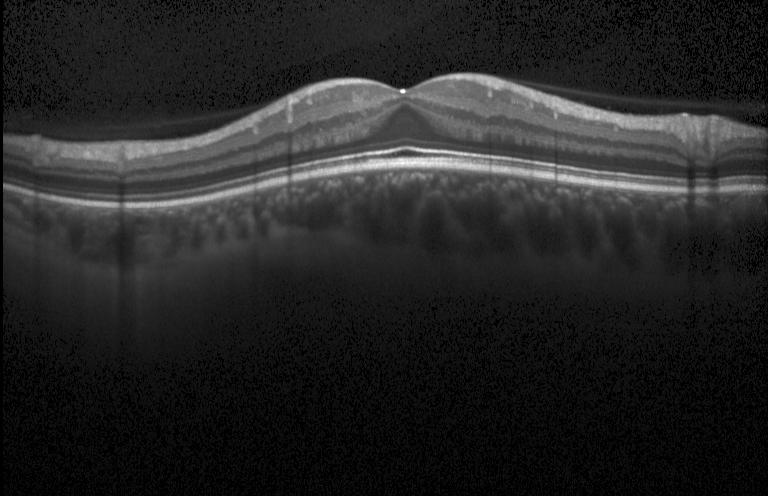 Dx: no choroidal neovascularization, diabetic macular edema, or drusen.